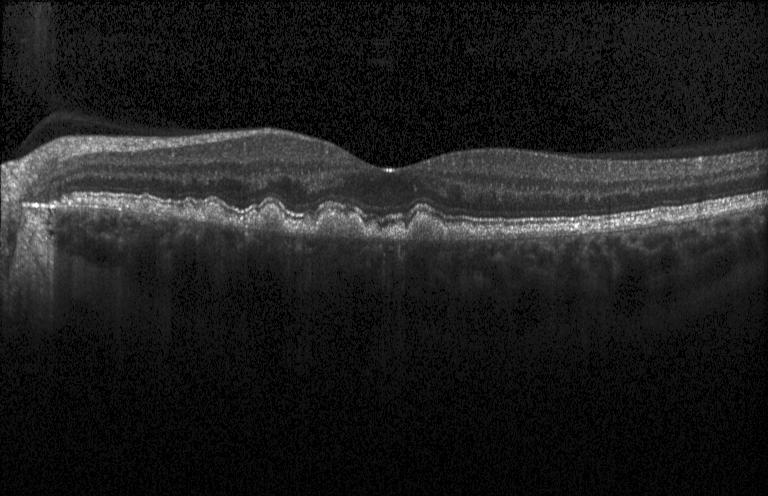
Instrument: Heidelberg Spectralis · spectral-domain optical coherence tomography · OCT line scan · centered on the fovea.
Diagnosis: sub-RPE drusenoid deposits.